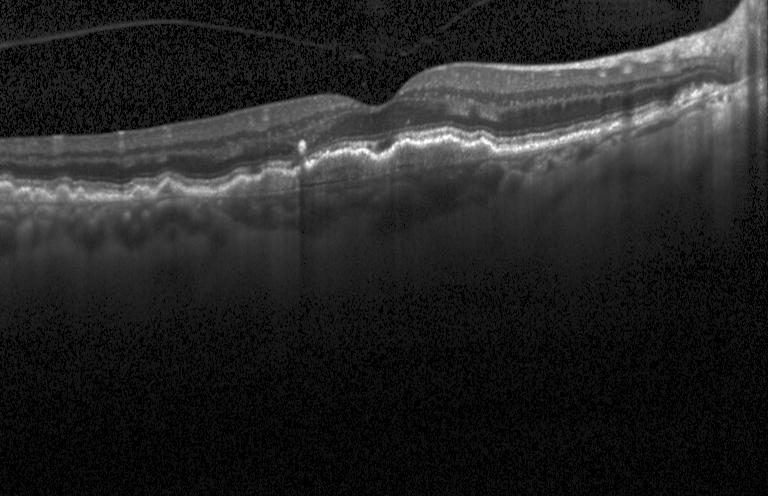

Retinal OCT B-scan — Dx: CNV.